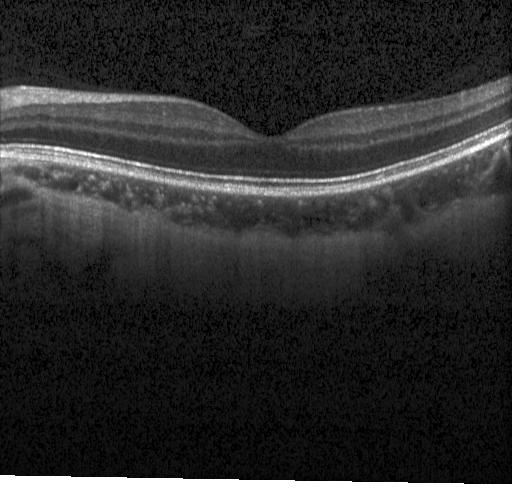
Neither choroidal neovascularization, diabetic macular edema, nor drusen.